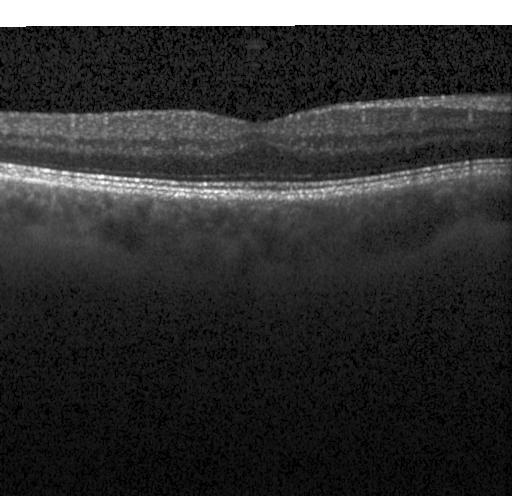 Finding: no evidence of choroidal neovascularization, diabetic macular edema, or drusen.